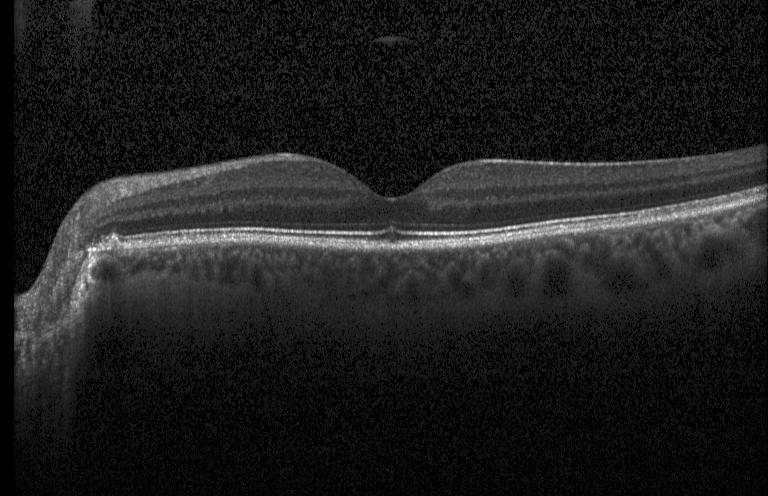 Finding: no choroidal neovascularization, diabetic macular edema, or drusen.